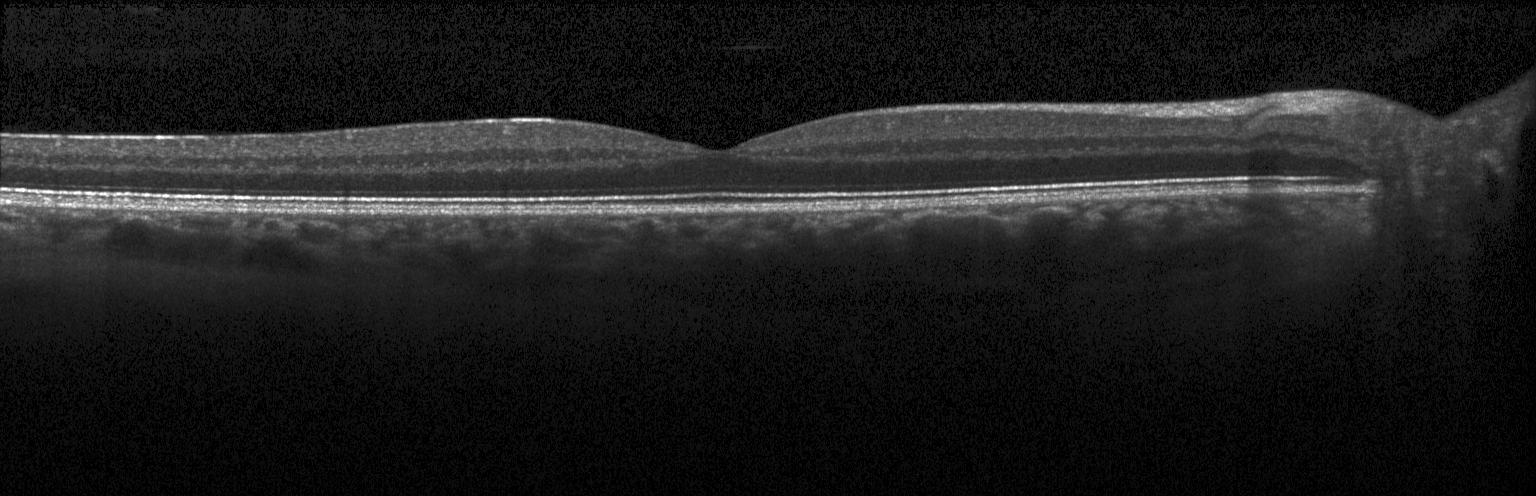

Instrument: Heidelberg Spectralis · spectral-domain optical coherence tomography · OCT B-scan · fovea-centered. OCT finding: no evidence of choroidal neovascularization, diabetic macular edema, or drusen.